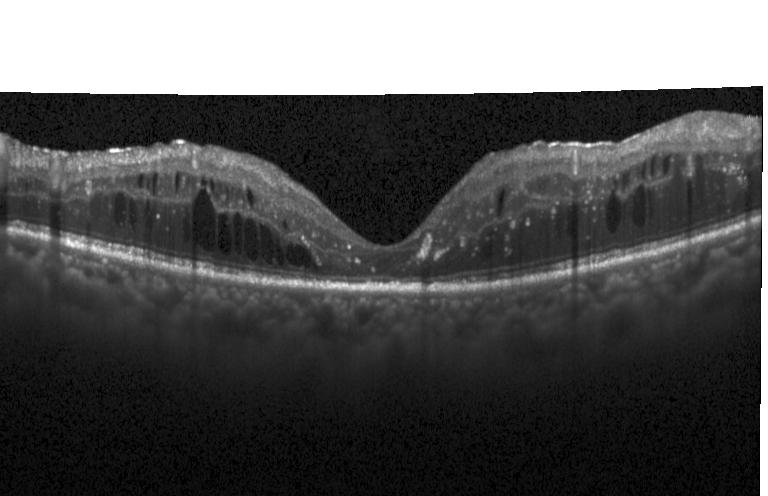 OCT finding: diabetic macular edema.